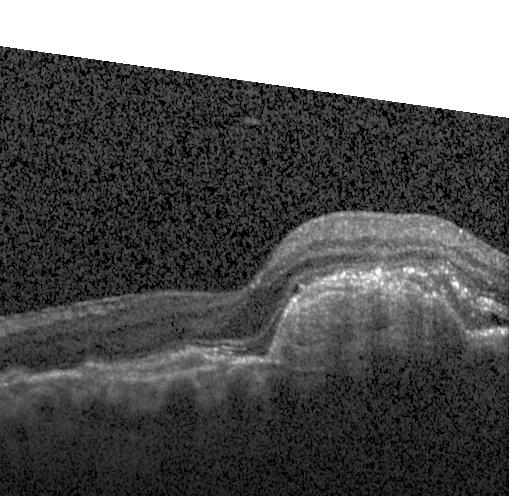 Finding: choroidal neovascularization (CNV).